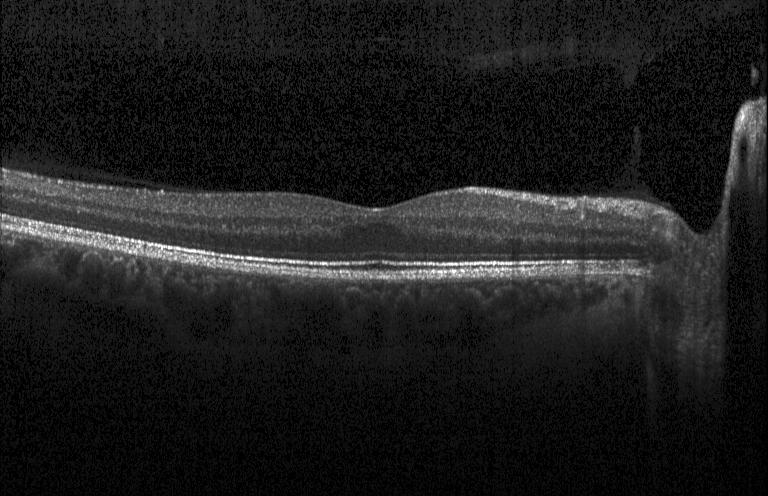
OCT line scan
Assessment: no choroidal neovascularization, no diabetic macular edema, and no drusen.